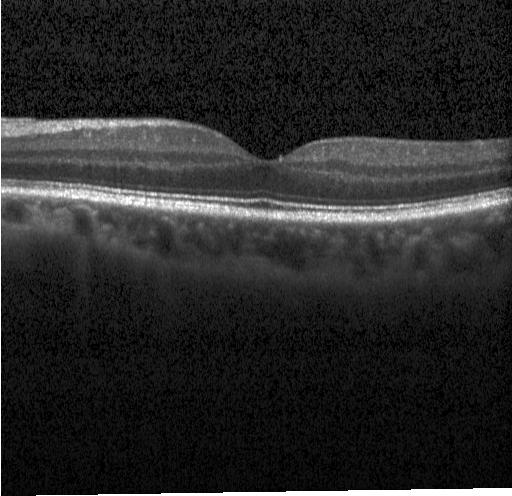

This B-scan demonstrates neither CNV, DME, nor drusen.